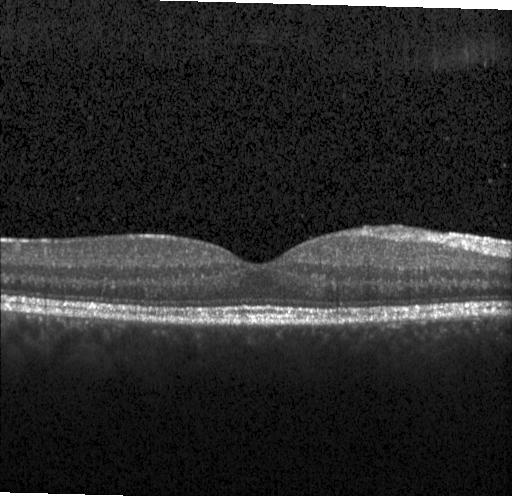

Retinal OCT B-scan. OCT finding: no evidence of CNV, DME, or drusen.